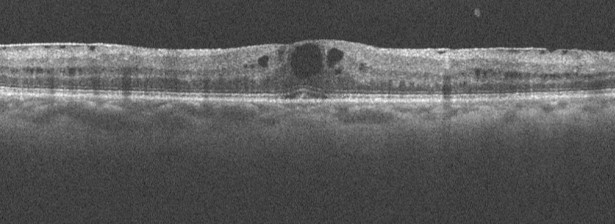

Dx: diabetic macular edema.